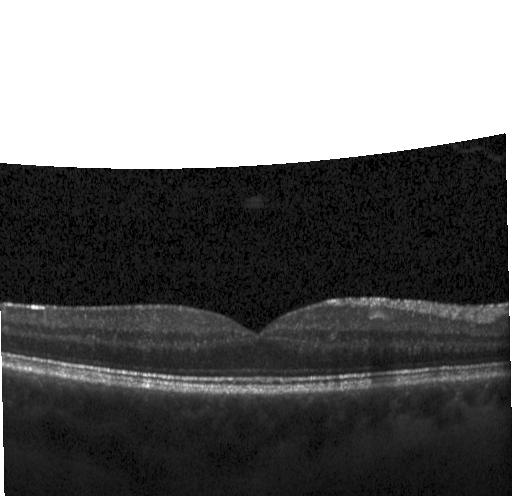 Macular OCT: neither choroidal neovascularization, diabetic macular edema, nor drusen.